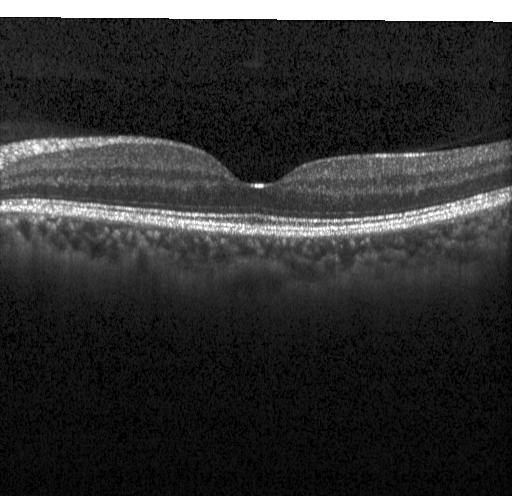 Finding: neither CNV, DME, nor drusen.